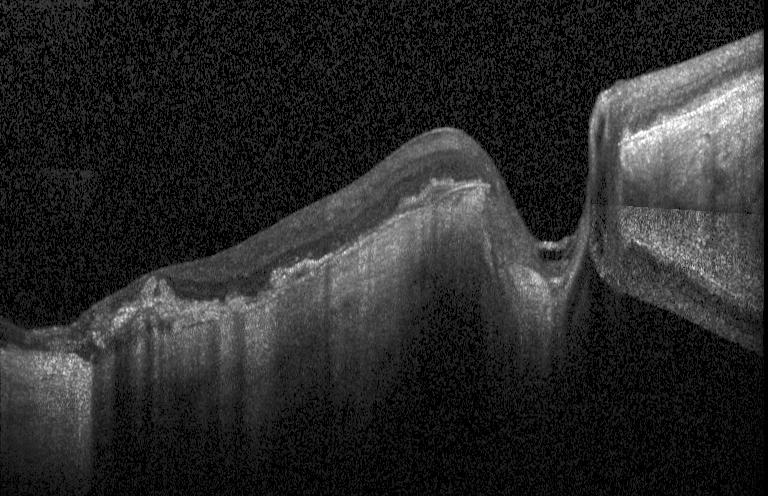 Spectral-domain optical coherence tomography; acquired on a Heidelberg Spectralis; retinal OCT B-scan; horizontal scan through the fovea
Finding: a choroidal neovascular membrane.